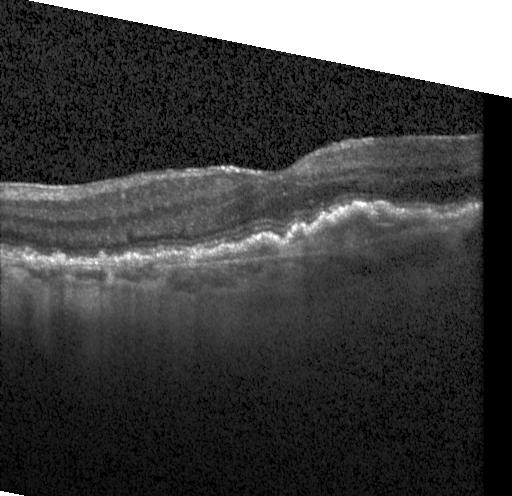

Retinal OCT B-scan.
Finding: CNV.